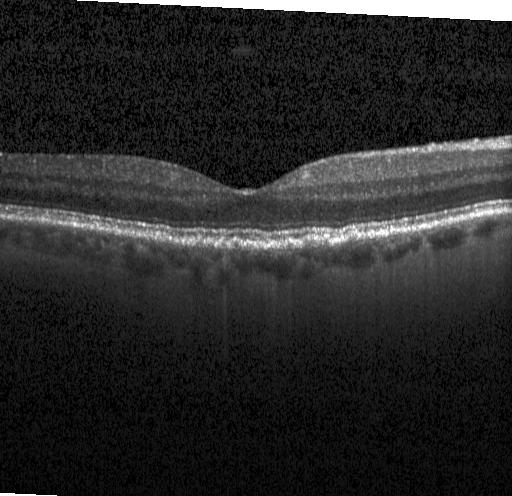
Retinal OCT B-scan · Heidelberg Spectralis. Finding: multiple drusen.